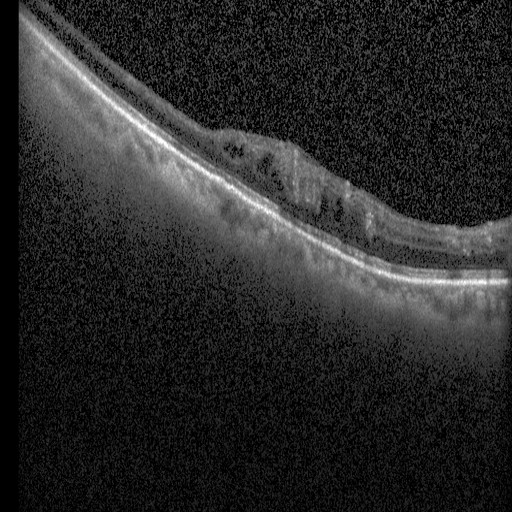

Macular OCT: diabetic macular edema (DME).